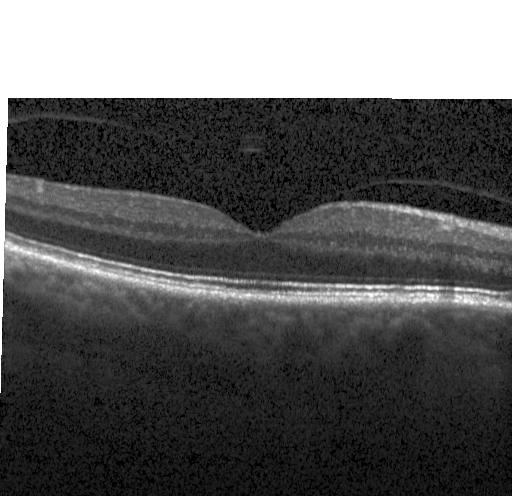

Heidelberg Spectralis OCT system · SD-OCT · optical coherence tomography scan · centered on the fovea
The scan shows no evidence of CNV, DME, or drusen.